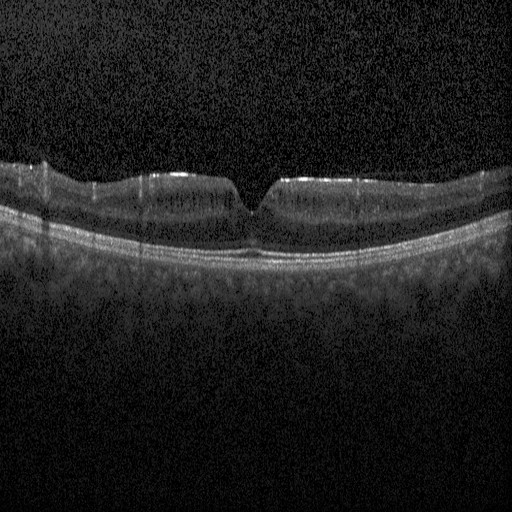 Through the macula. Retinal OCT B-scan.
Assessment: diabetic macular edema.